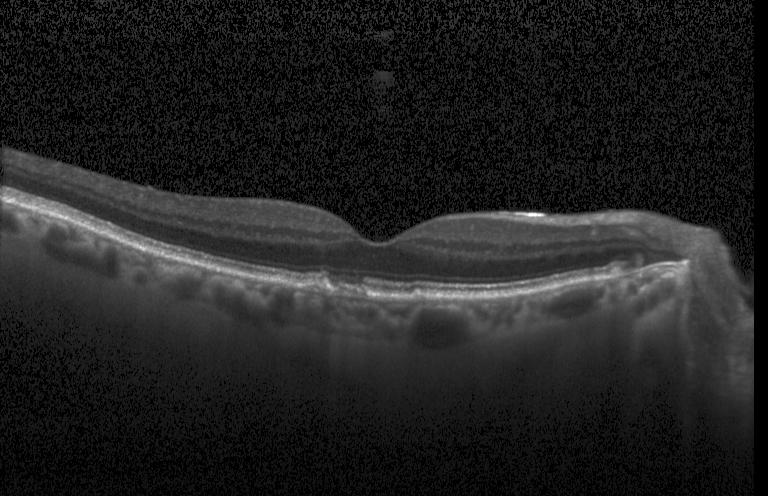

Retinal OCT B-scan.
Assessment: sub-RPE drusenoid deposits.